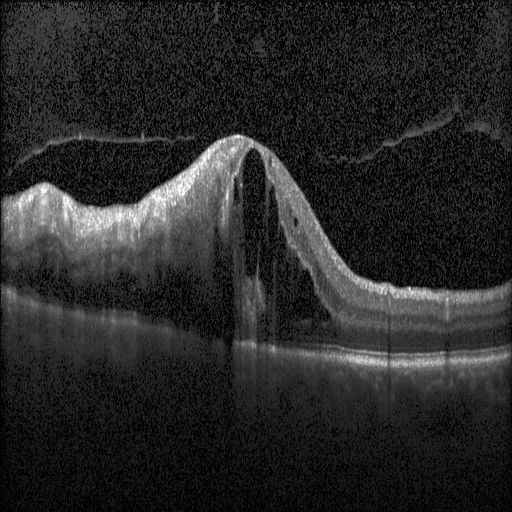
Retinal OCT B-scan, Heidelberg Spectralis OCT system, spectral-domain optical coherence tomography, fovea-centered. Impression: diabetic macular edema (DME).